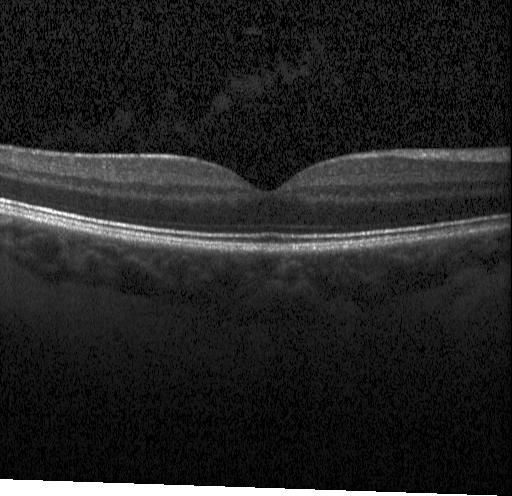
Centered on the fovea. Heidelberg Spectralis. OCT line scan. SD-OCT.
Diagnosis: no evidence of choroidal neovascularization, diabetic macular edema, or drusen.